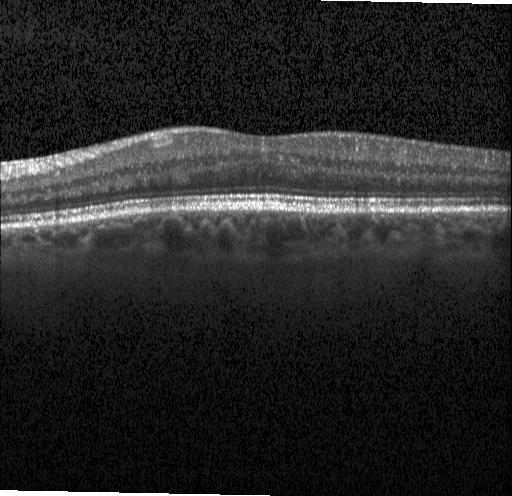 Heidelberg Spectralis OCT system · retinal OCT cross-section. Finding: no choroidal neovascularization, diabetic macular edema, or drusen.